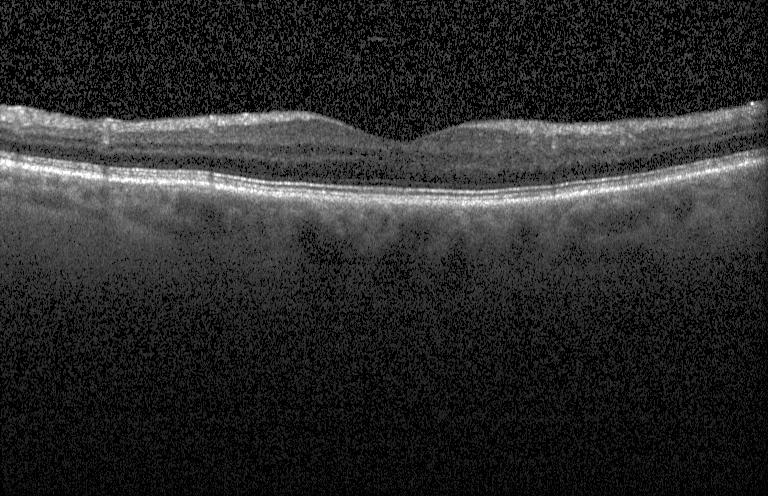
Spectral-domain OCT B-scan: no choroidal neovascularization, no diabetic macular edema, and no drusen.